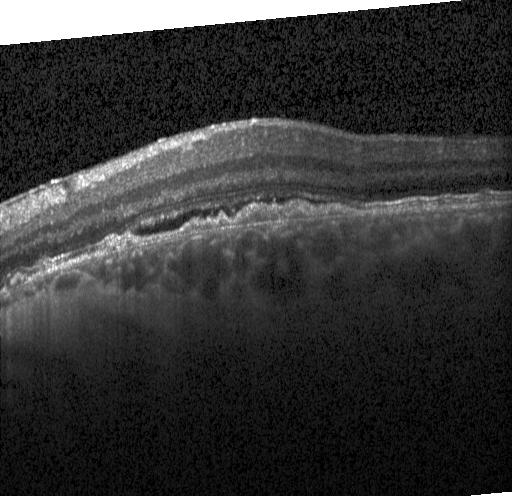
Diagnosis: choroidal neovascularization (CNV).